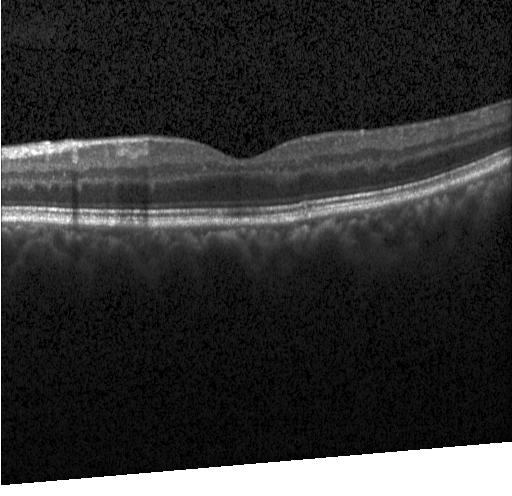
Finding: no choroidal neovascularization, no diabetic macular edema, and no drusen.